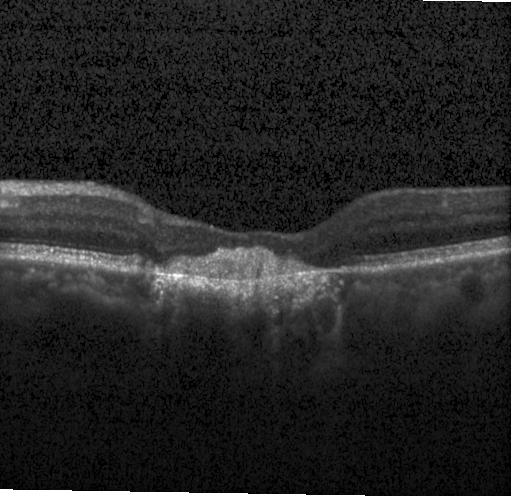 OCT line scan
Diagnosis: choroidal neovascularization.